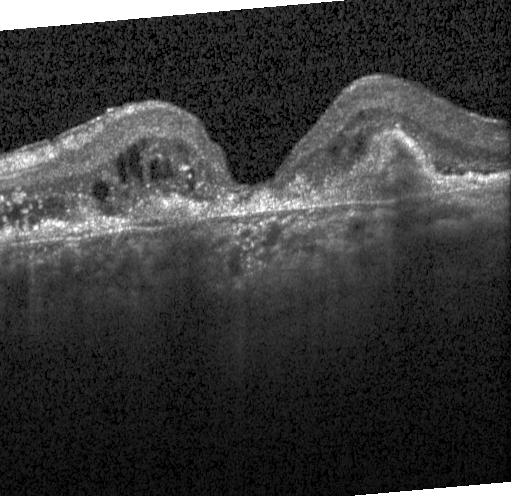
Dx: a choroidal neovascular membrane.